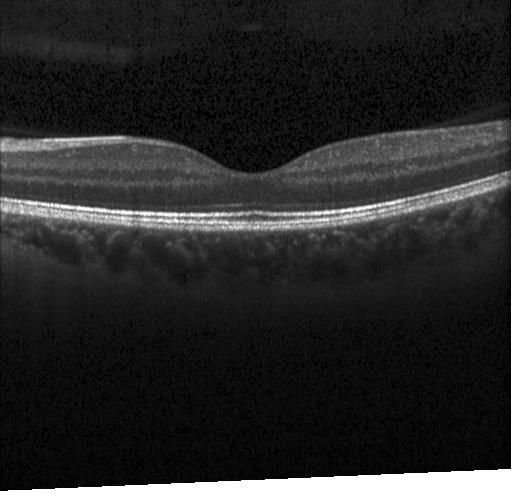
Retinal OCT cross-section showing no evidence of CNV, DME, or drusen.